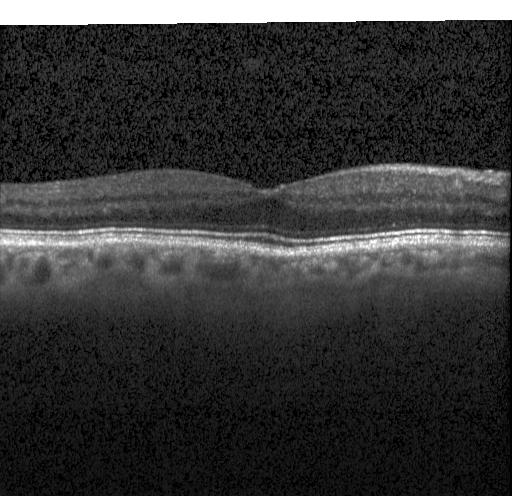
The scan shows no choroidal neovascularization, no diabetic macular edema, and no drusen.